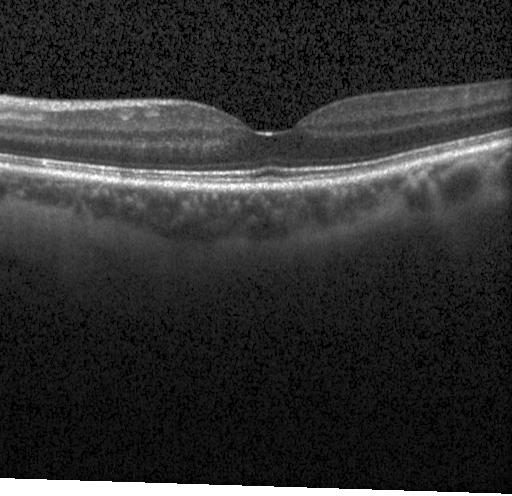
Neither choroidal neovascularization, diabetic macular edema, nor drusen.